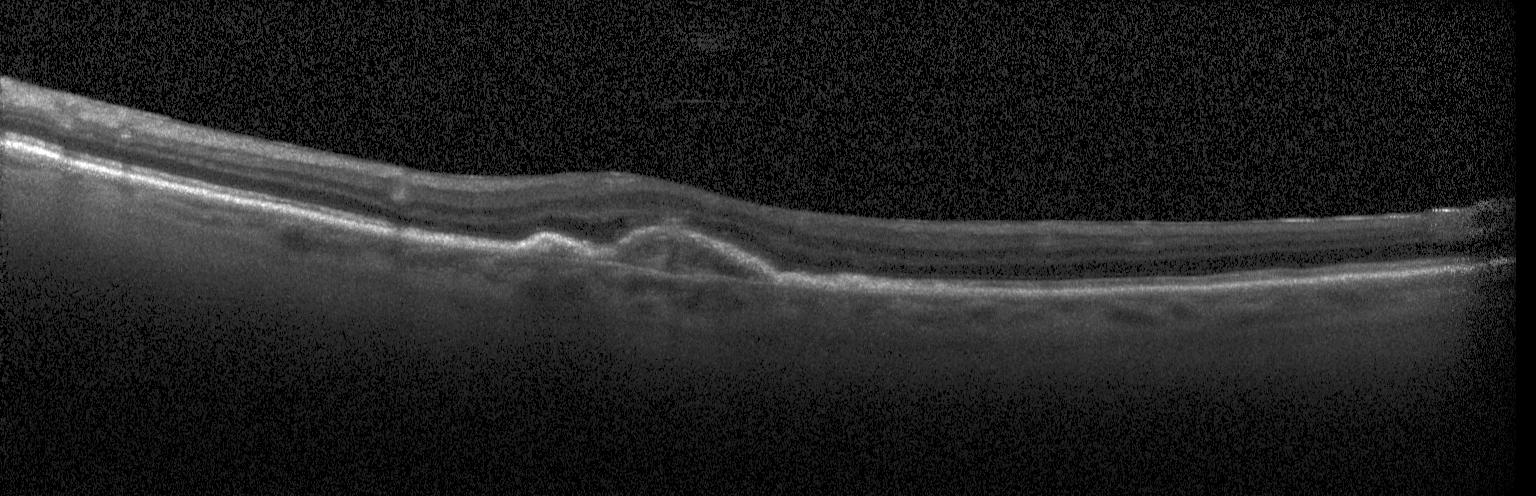
Macular scan; retinal OCT cross-section.
Finding: choroidal neovascularization.